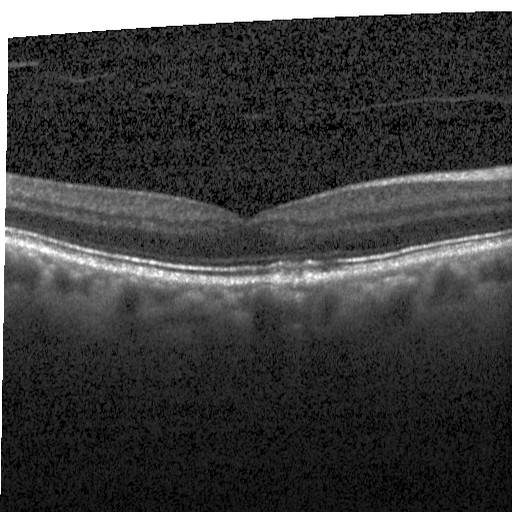
OCT B-scan showing DME.